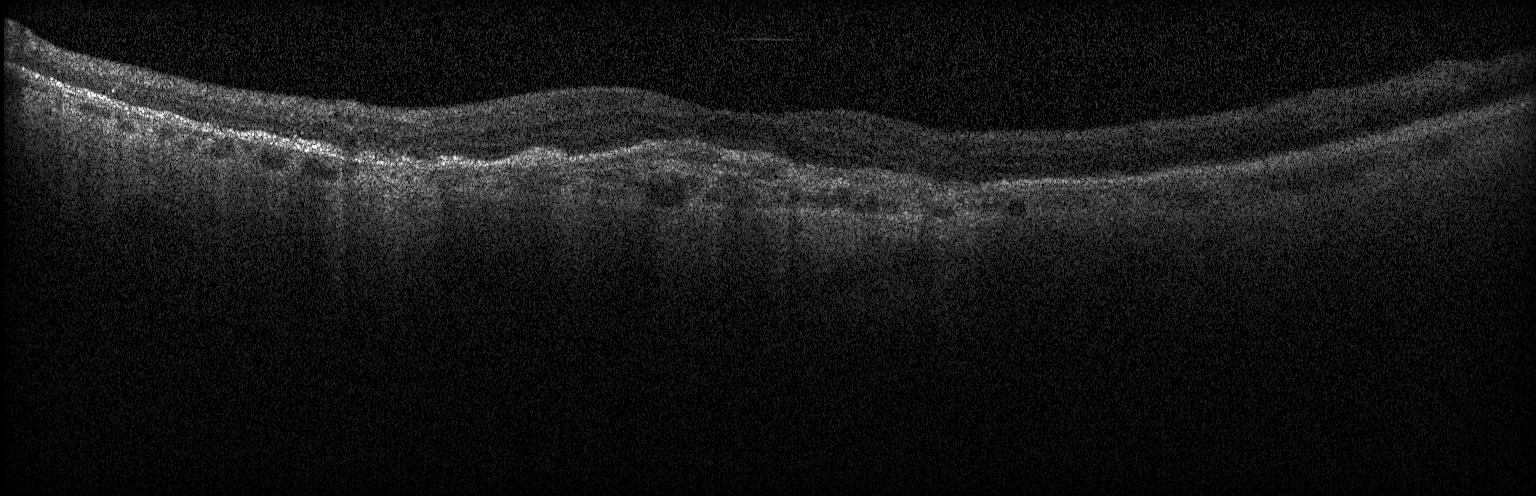

Heidelberg Spectralis OCT system; horizontal scan through the fovea; OCT line scan — Dx: a choroidal neovascular membrane.